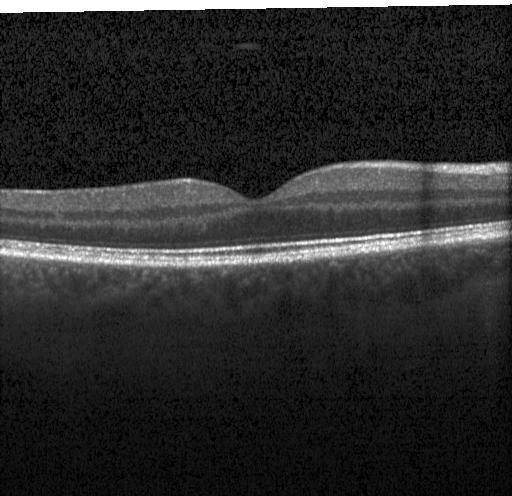 Macular scan. SD-OCT. Retinal OCT B-scan. Heidelberg Spectralis — Finding: no evidence of choroidal neovascularization, diabetic macular edema, or drusen.